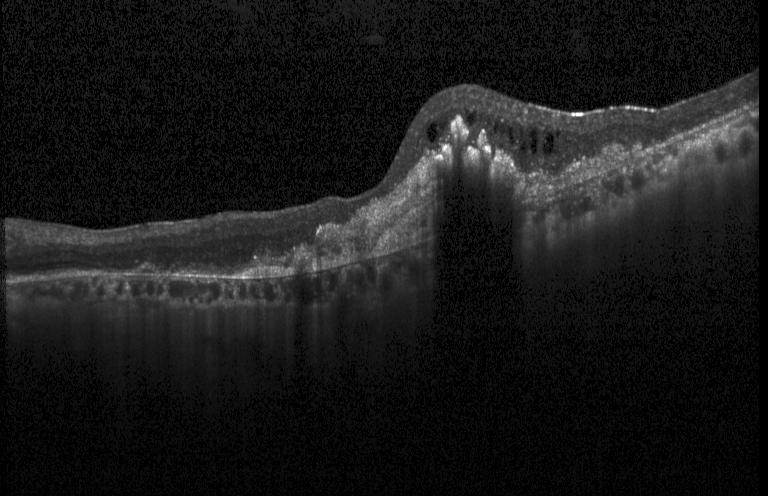
Impression: a choroidal neovascular membrane.